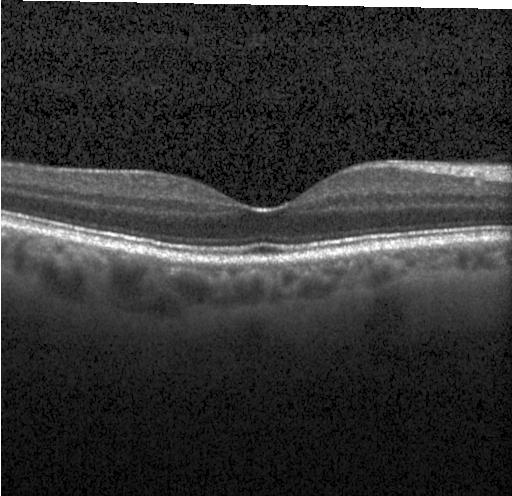
Through the macula · instrument: Heidelberg Spectralis · optical coherence tomography B-scan · spectral-domain optical coherence tomography
Assessment: no choroidal neovascularization, diabetic macular edema, or drusen.